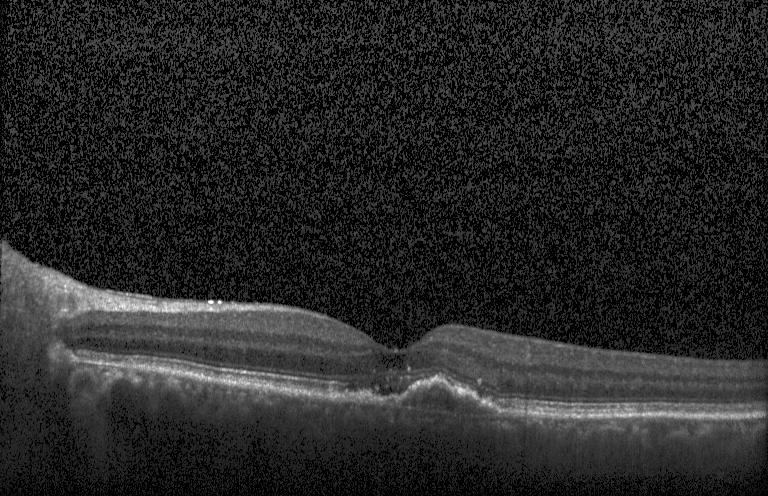

Heidelberg Spectralis · through the macula · OCT B-scan. Assessment: a choroidal neovascular membrane.